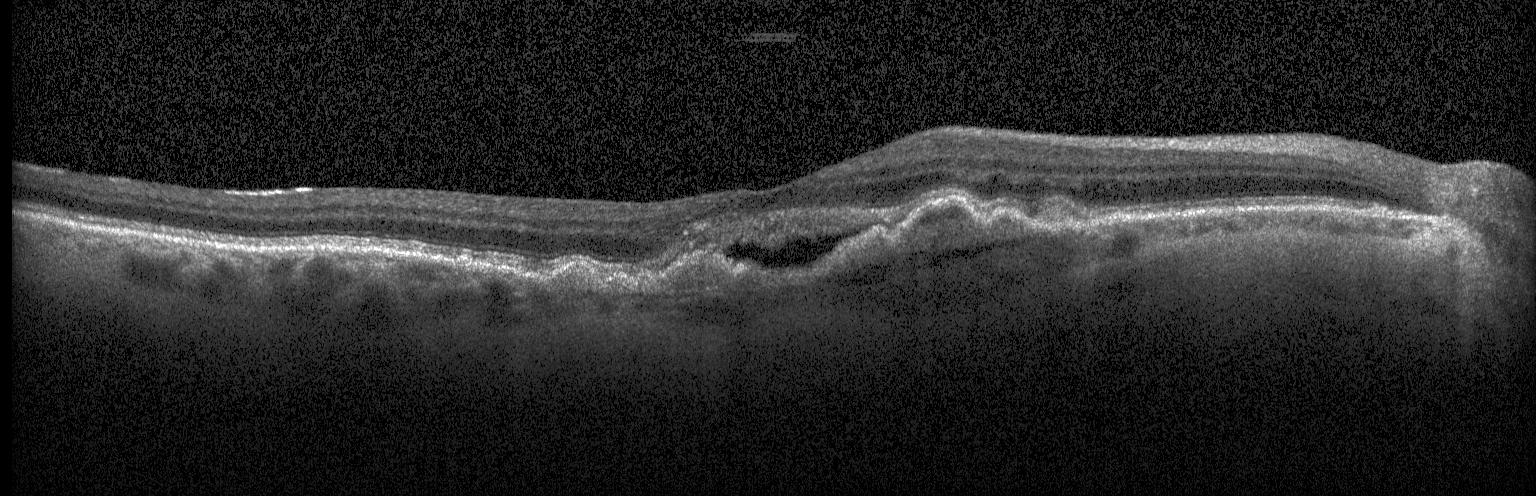
OCT B-scan; spectral-domain OCT; Heidelberg Spectralis OCT system; centered on the fovea
The scan shows CNV.